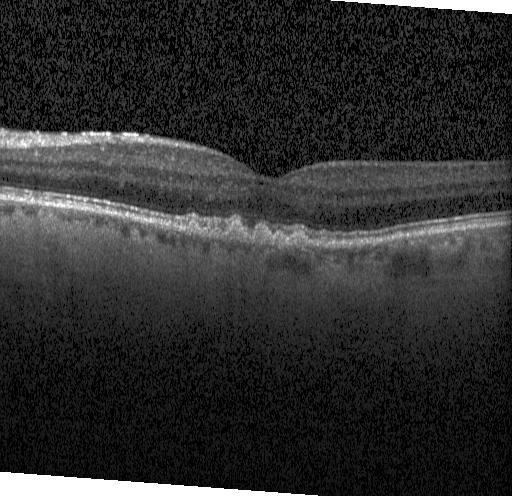
OCT B-scan
Impression: drusen.